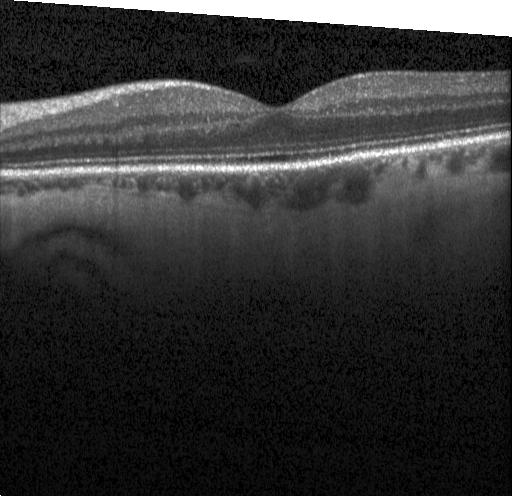
Spectral-domain optical coherence tomography · optical coherence tomography B-scan. Impression: no choroidal neovascularization, no diabetic macular edema, and no drusen.